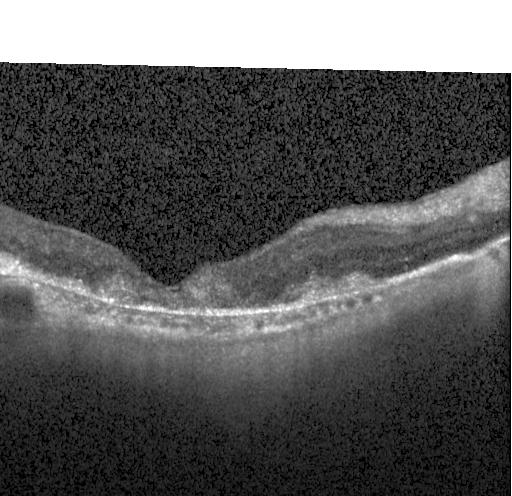 Heidelberg Spectralis OCT system · spectral-domain OCT · retinal OCT B-scan · macular scan — Macular OCT: CNV.